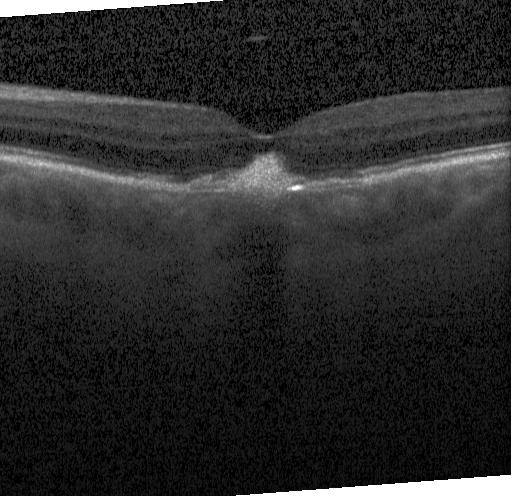

Retinal OCT B-scan
Finding: choroidal neovascularization (CNV).